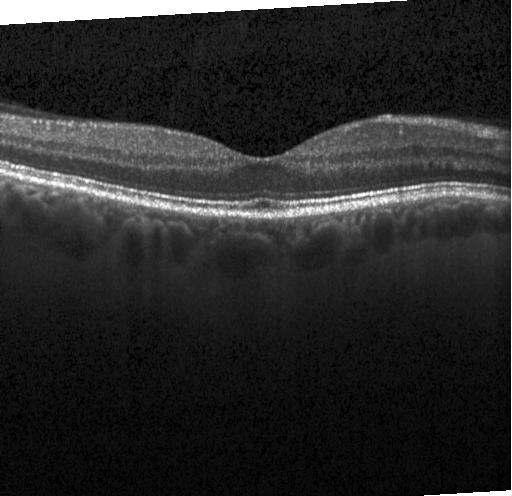
Finding: no evidence of CNV, DME, or drusen.